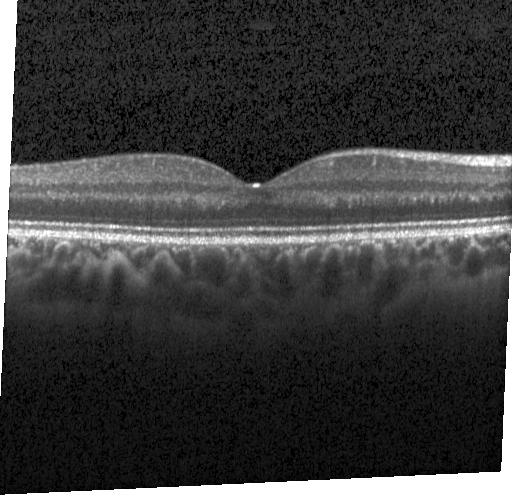 OCT B-scan. SD-OCT. Instrument: Heidelberg Spectralis.
This B-scan demonstrates no CNV, no DME, and no drusen.